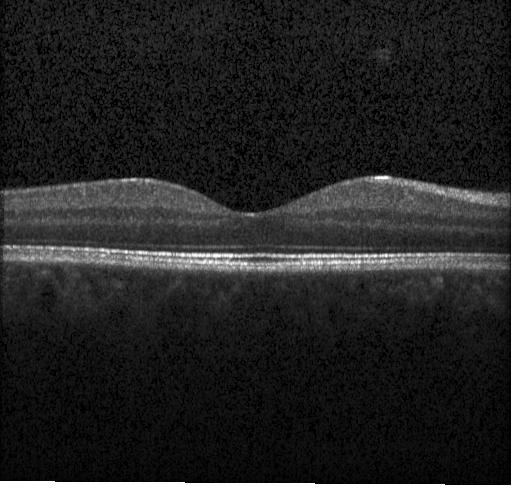 Dx: no CNV, no DME, and no drusen.